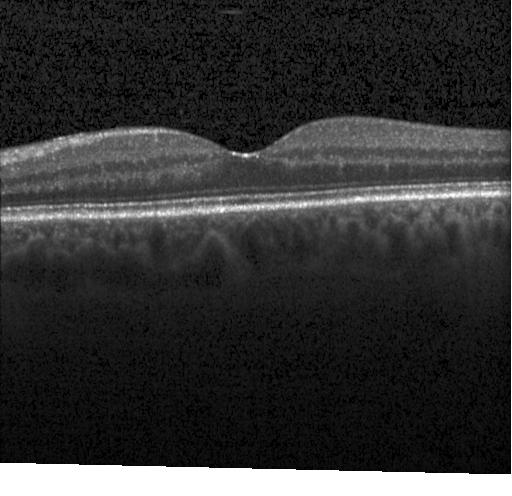 Centered on the fovea; optical coherence tomography B-scan; Heidelberg Spectralis OCT system
Diagnosis: no choroidal neovascularization, diabetic macular edema, or drusen.